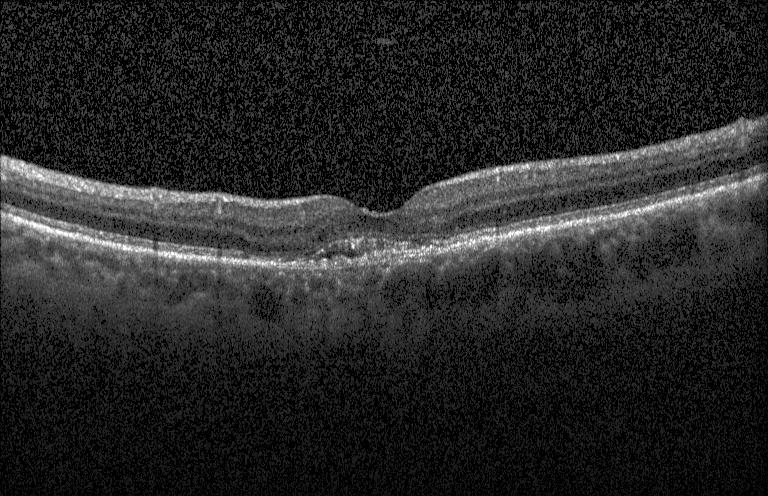

Retinal OCT cross-section showing choroidal neovascularization (CNV).